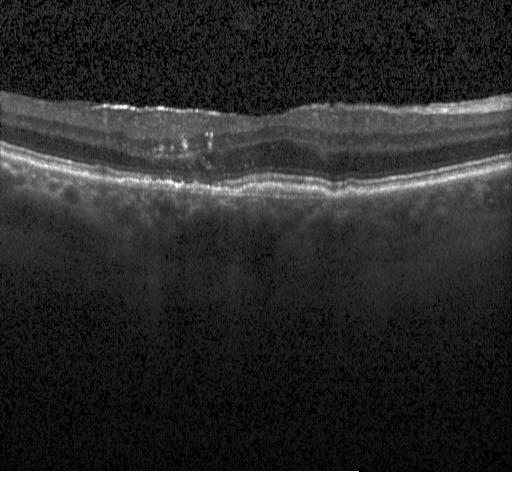 Spectral-domain OCT · OCT line scan — Dx: choroidal neovascularization (CNV).